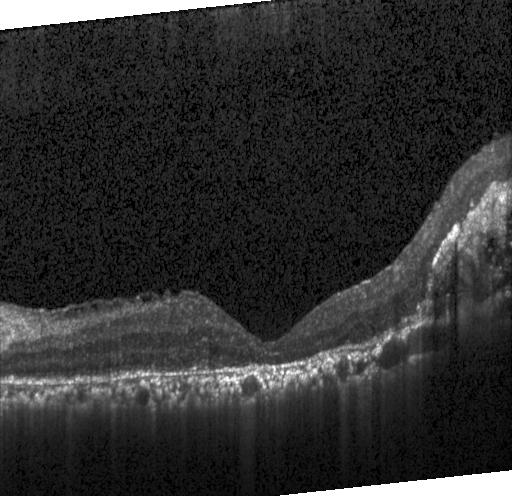 Optical coherence tomography B-scan · macular scan. Macular OCT: a choroidal neovascular membrane.